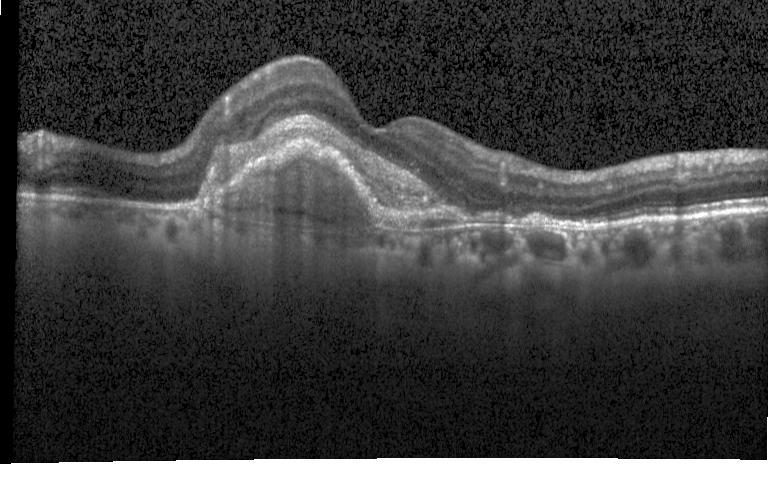
Spectral-domain OCT, centered on the fovea, acquired on a Heidelberg Spectralis, optical coherence tomography B-scan. Finding: choroidal neovascularization (CNV).